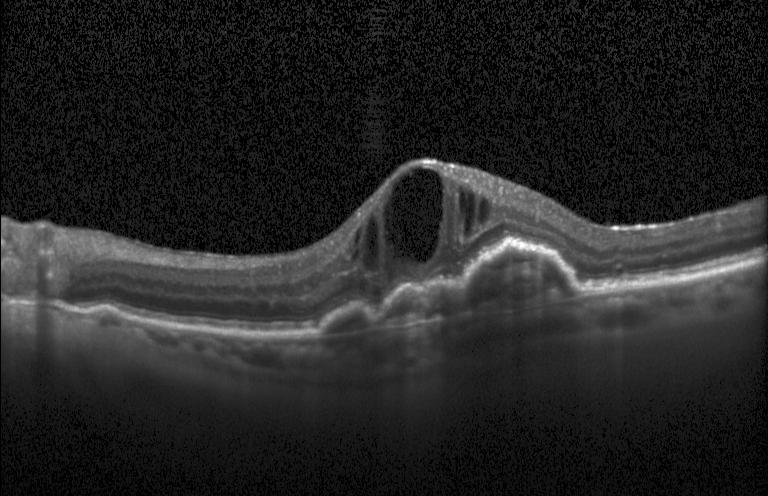
Optical coherence tomography scan
Impression: choroidal neovascularization (CNV).